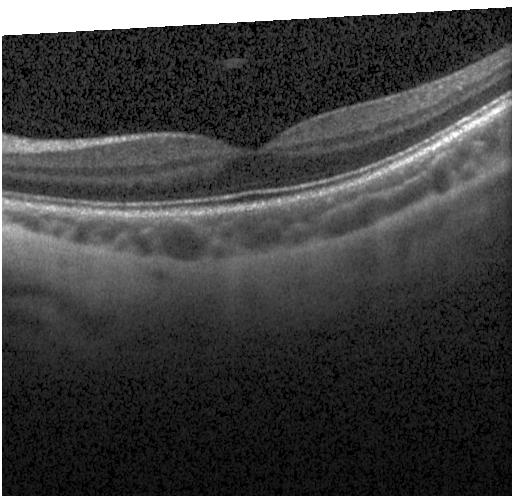

Optical coherence tomography scan
Dx: neither choroidal neovascularization, diabetic macular edema, nor drusen.